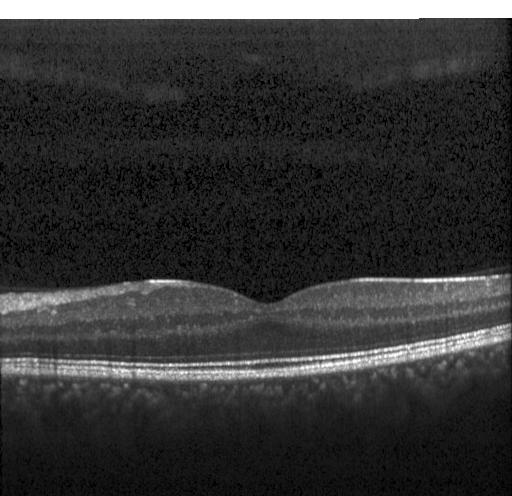 Through the macula; Heidelberg Spectralis OCT system; retinal OCT cross-section. Finding: no choroidal neovascularization, diabetic macular edema, or drusen.